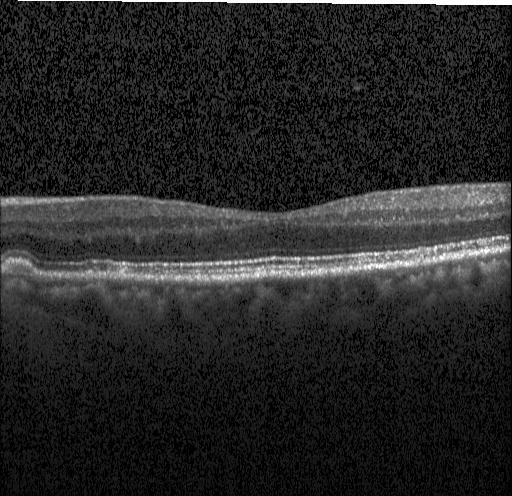 Retinal OCT B-scan · Heidelberg Spectralis OCT system · spectral-domain OCT · macular scan. This B-scan demonstrates sub-RPE drusenoid deposits.